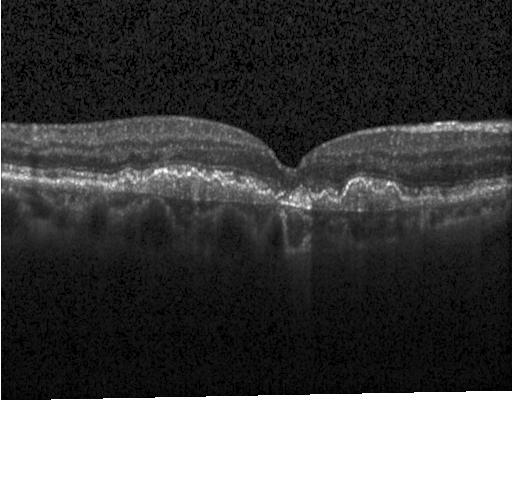
Macular OCT demonstrating a choroidal neovascular membrane.